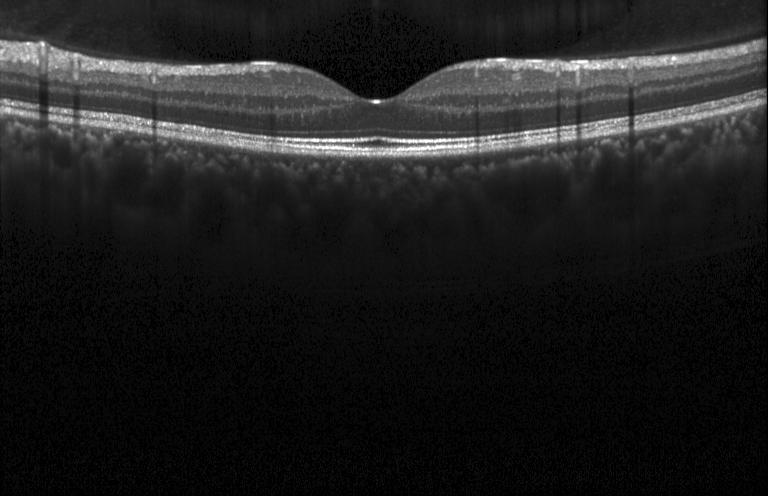 Impression: no evidence of choroidal neovascularization, diabetic macular edema, or drusen.